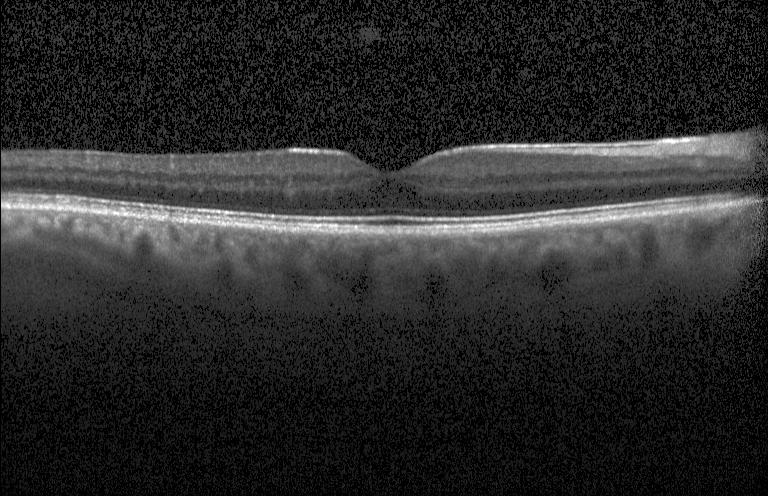
OCT finding: neither choroidal neovascularization, diabetic macular edema, nor drusen.